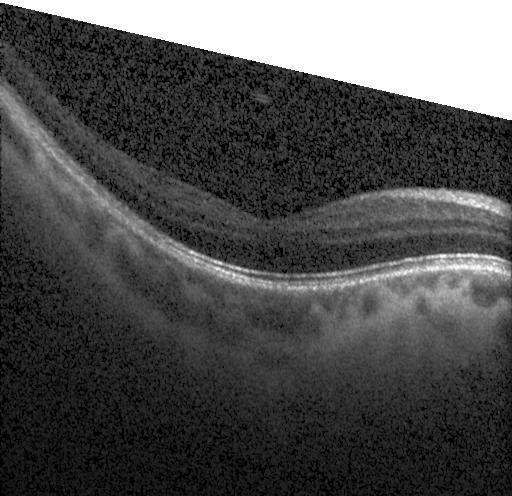 Impression: no choroidal neovascularization, diabetic macular edema, or drusen.